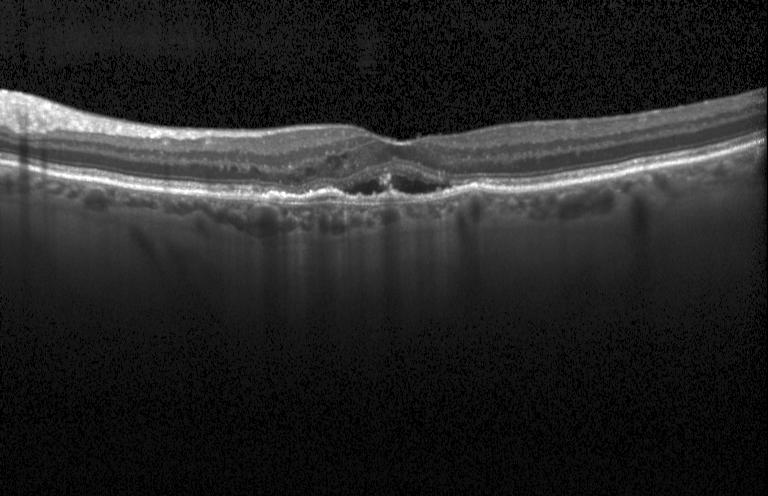

Macular OCT demonstrating a choroidal neovascular membrane.